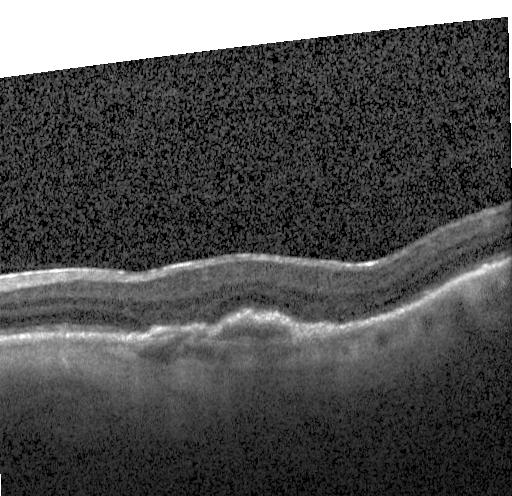

Optical coherence tomography B-scan · centered on the fovea · instrument: Heidelberg Spectralis — The scan shows choroidal neovascularization (CNV).